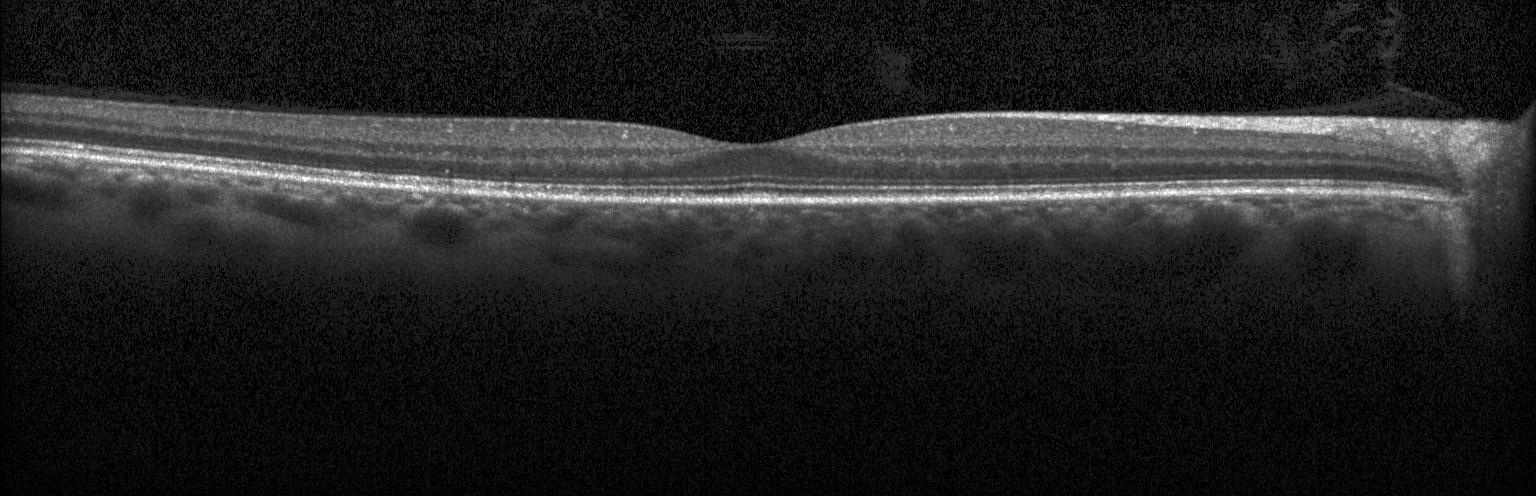
Macular OCT: no CNV, no DME, and no drusen.